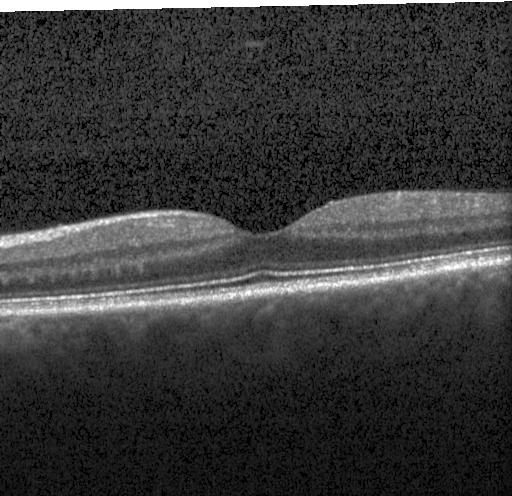

Through the macula; spectral-domain optical coherence tomography; retinal OCT cross-section
OCT finding: no choroidal neovascularization, diabetic macular edema, or drusen.